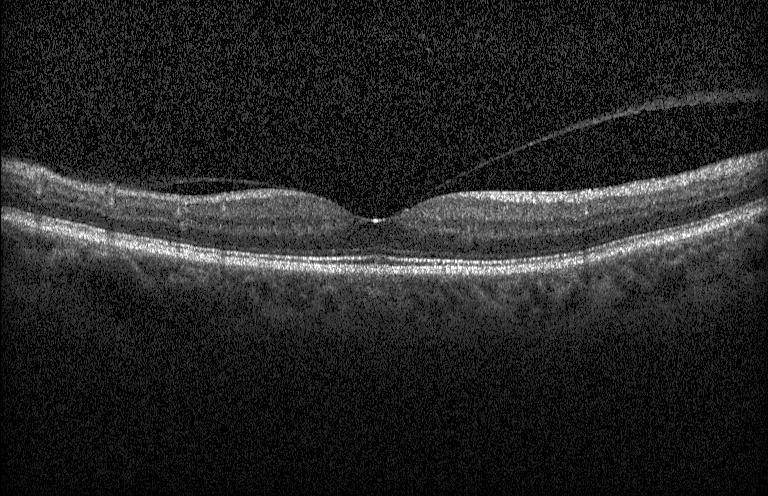

Macular OCT demonstrating no evidence of choroidal neovascularization, diabetic macular edema, or drusen.